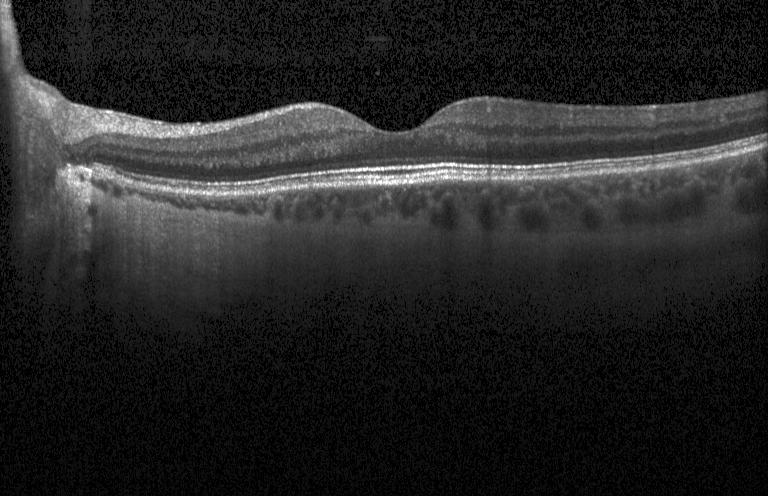
OCT line scan
Diagnosis: no evidence of choroidal neovascularization, diabetic macular edema, or drusen.